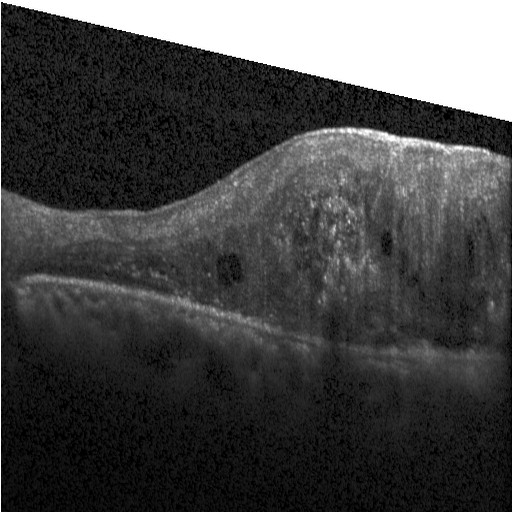
Impression: diabetic macular edema (DME).